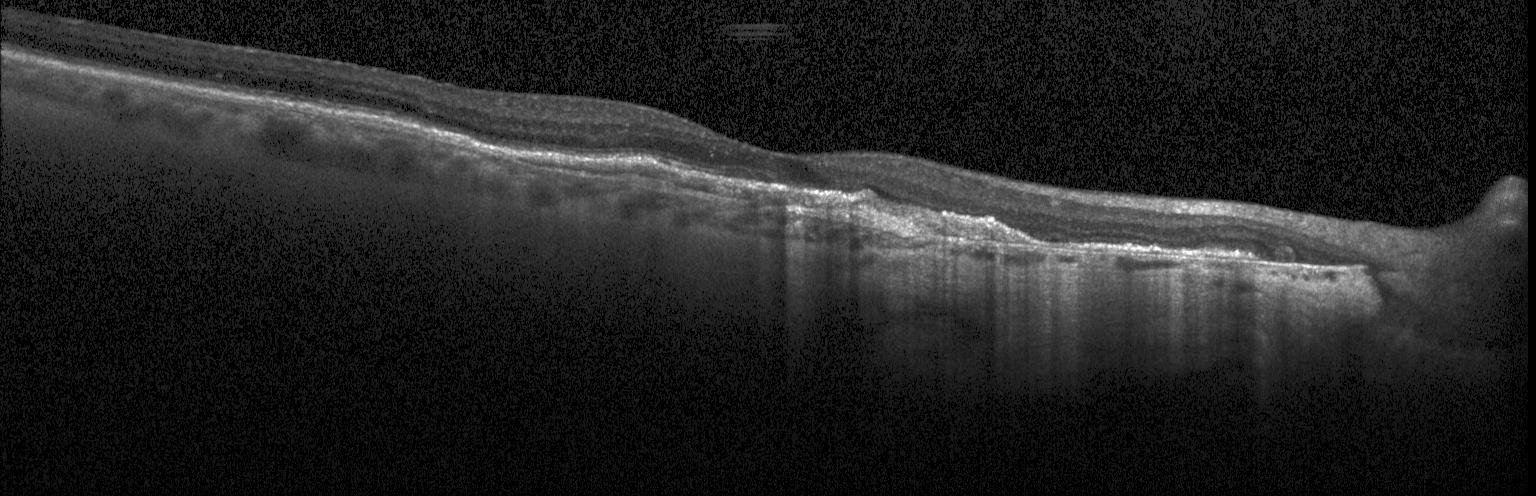

Finding: a choroidal neovascular membrane.